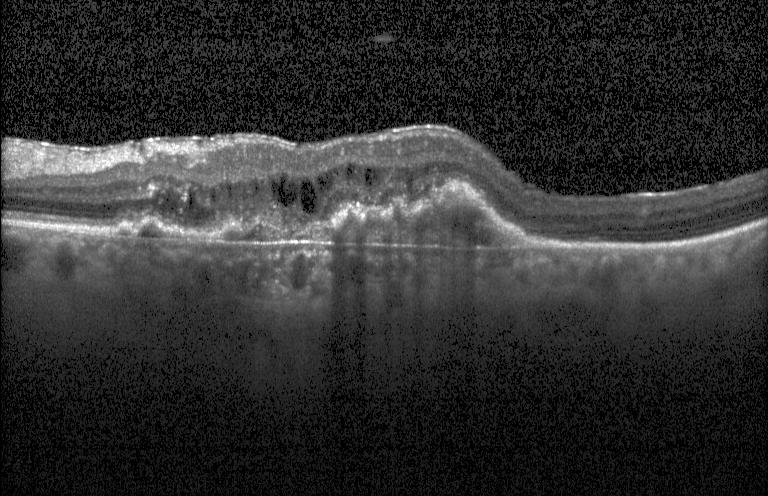

Retinal OCT cross-section · Heidelberg Spectralis OCT system — Dx: a choroidal neovascular membrane.